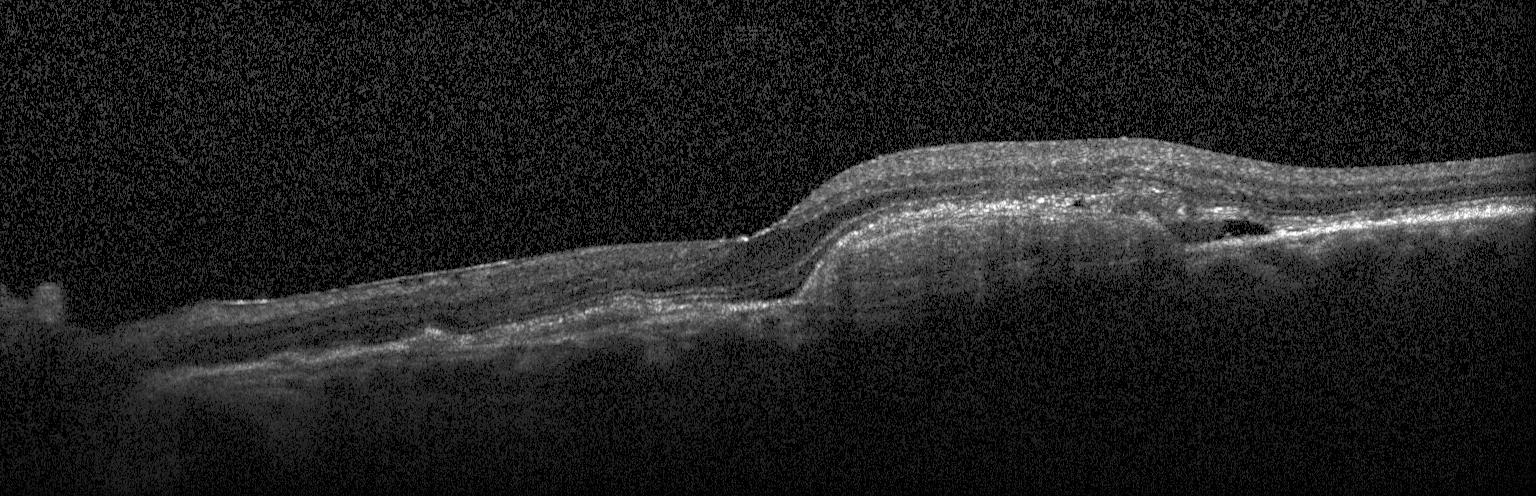
Diagnosis: choroidal neovascularization.